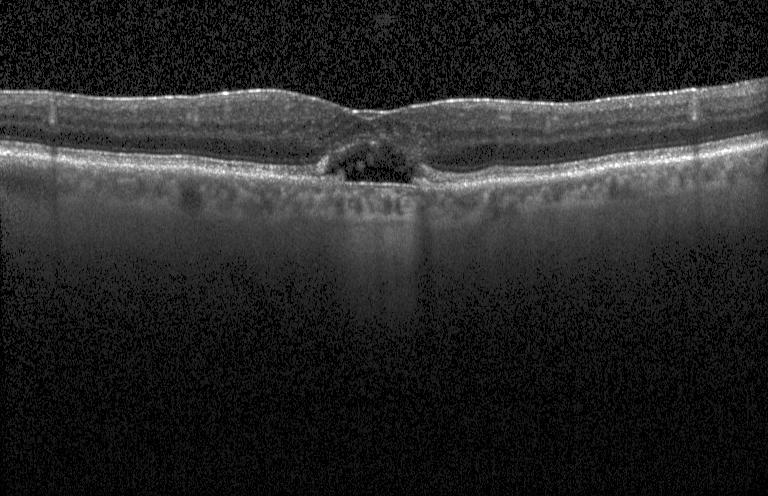
OCT finding: CNV.